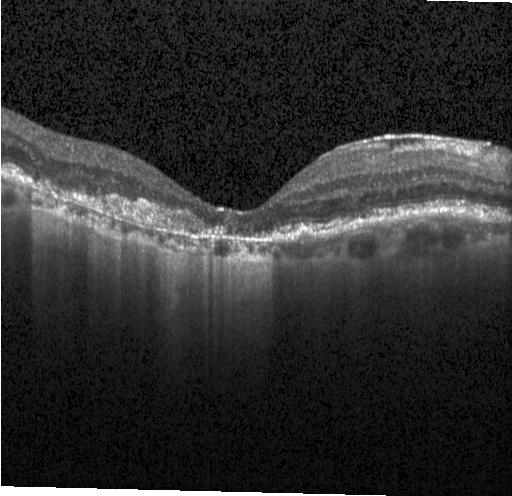
Horizontal scan through the fovea; instrument: Heidelberg Spectralis; retinal OCT B-scan; spectral-domain OCT
CNV.